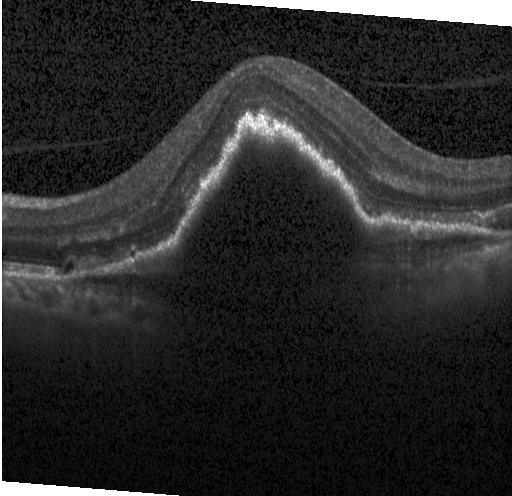 Retinal OCT cross-section — This B-scan demonstrates a choroidal neovascular membrane.